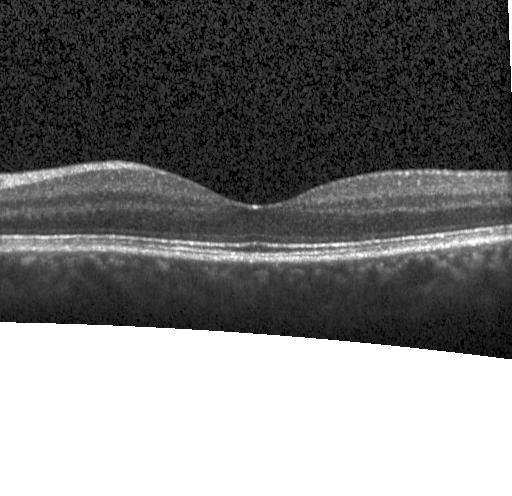

OCT B-scan — The scan shows neither choroidal neovascularization, diabetic macular edema, nor drusen.